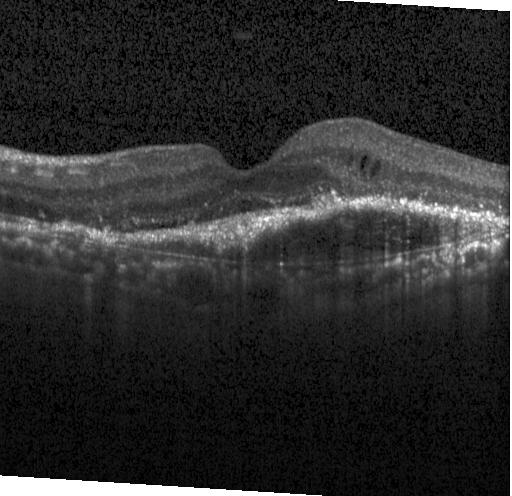
Retinal OCT cross-section.
This B-scan demonstrates choroidal neovascularization.